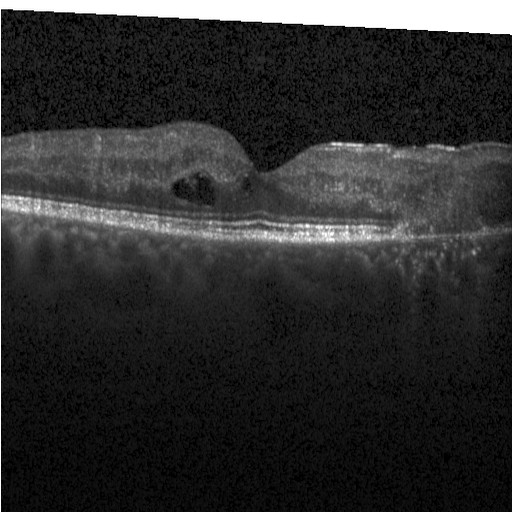 OCT B-scan showing diabetic macular edema (DME).